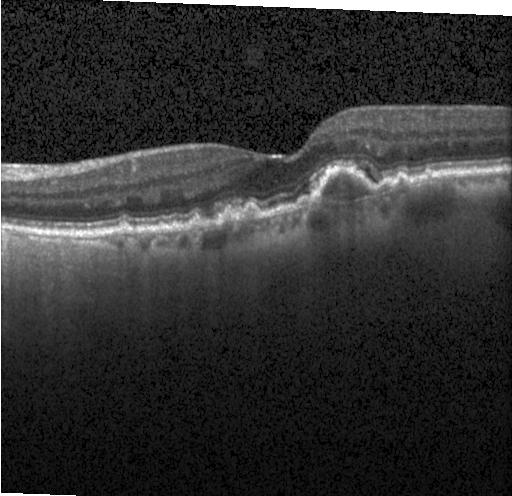 This B-scan demonstrates choroidal neovascularization (CNV).